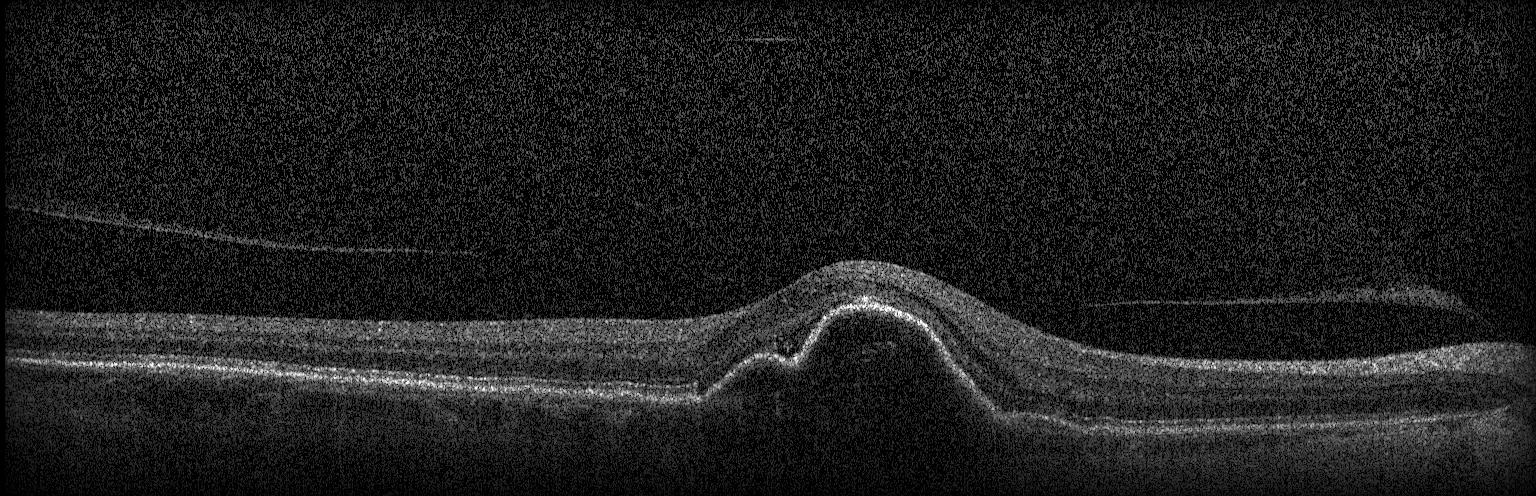

Assessment: choroidal neovascularization (CNV).